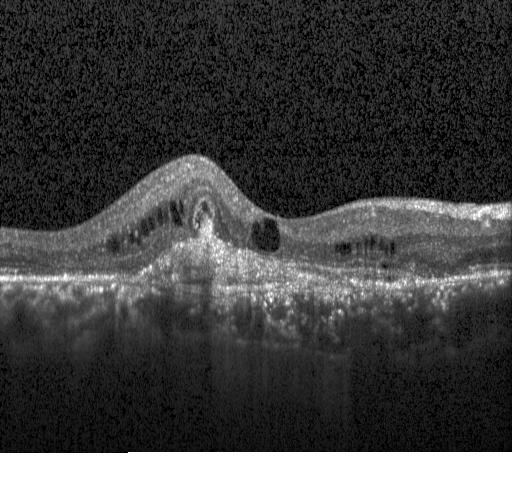 Spectral-domain OCT. Acquired on a Heidelberg Spectralis. Fovea-centered. OCT B-scan — This B-scan demonstrates choroidal neovascularization.